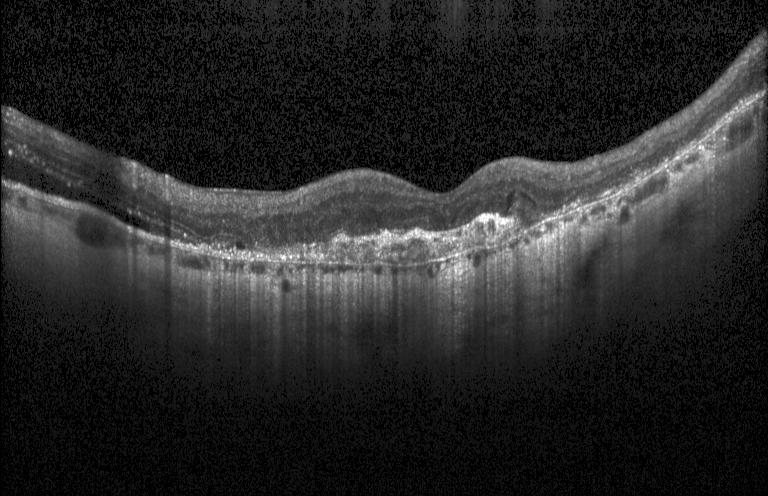
Fovea-centered; OCT B-scan — The scan shows CNV.